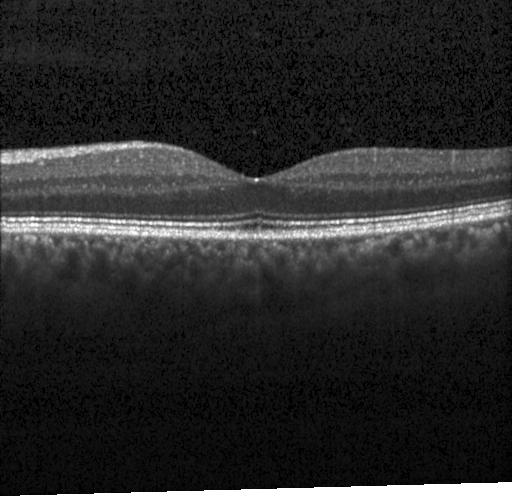 Dx: no choroidal neovascularization, diabetic macular edema, or drusen.